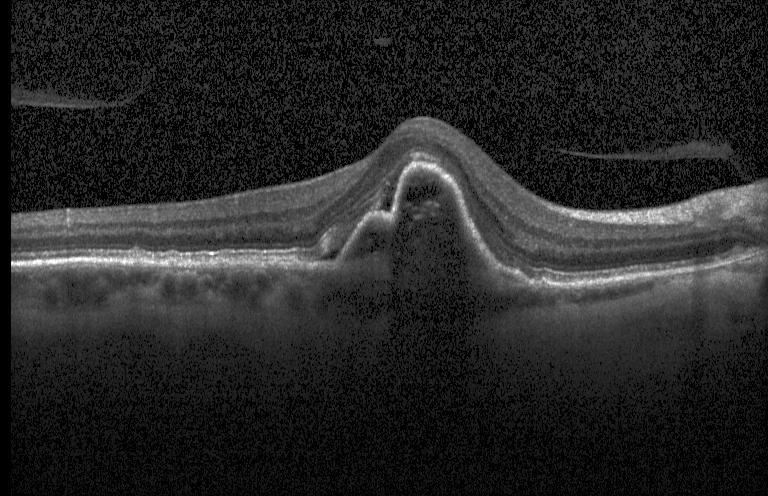

Retinal OCT cross-section; horizontal scan through the fovea
OCT finding: choroidal neovascularization (CNV).